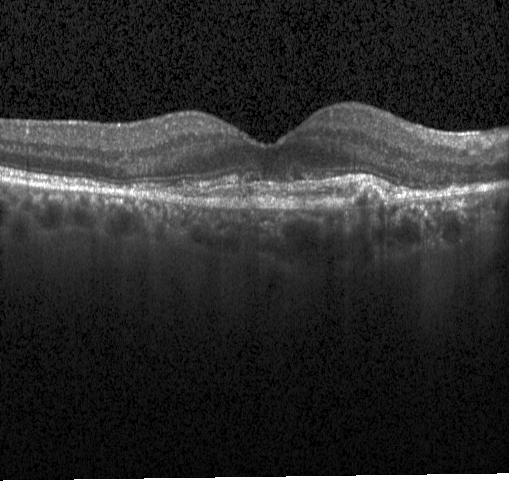
CNV.